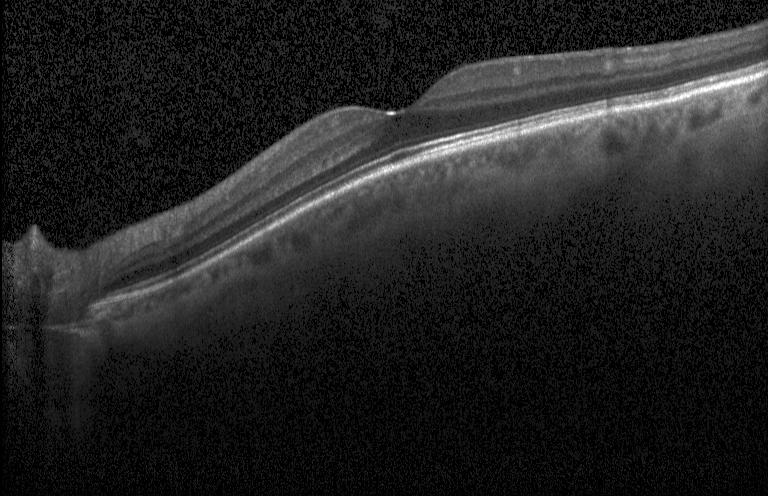

Macular OCT: no evidence of CNV, DME, or drusen.